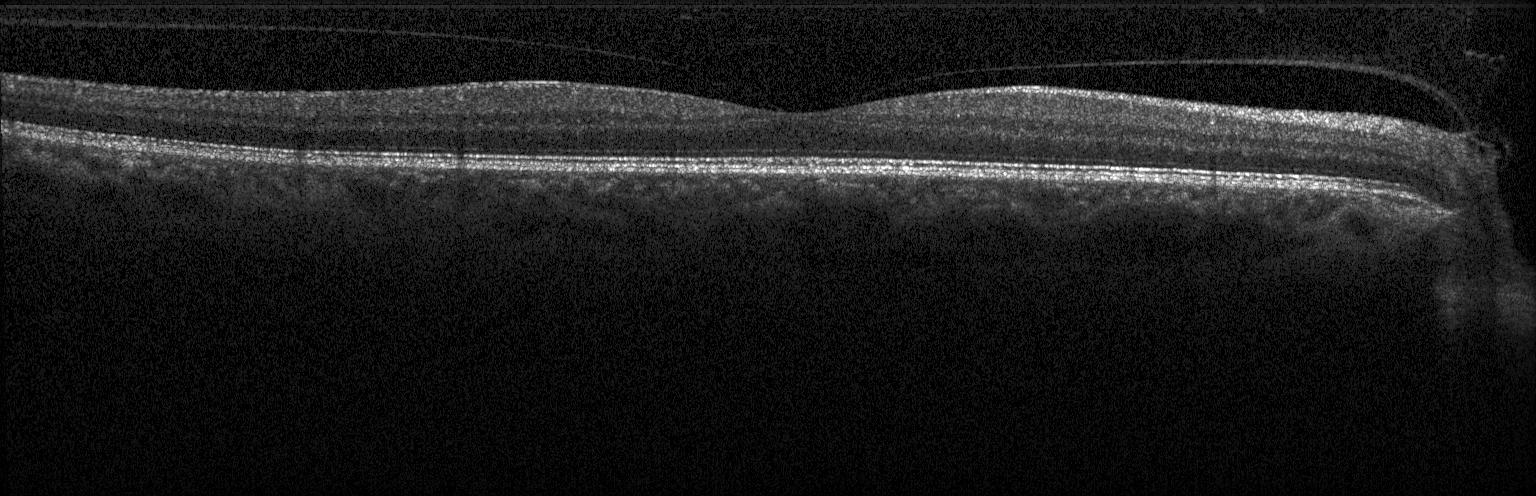
Optical coherence tomography scan, instrument: Heidelberg Spectralis, centered on the fovea — Macular OCT: no choroidal neovascularization, diabetic macular edema, or drusen.